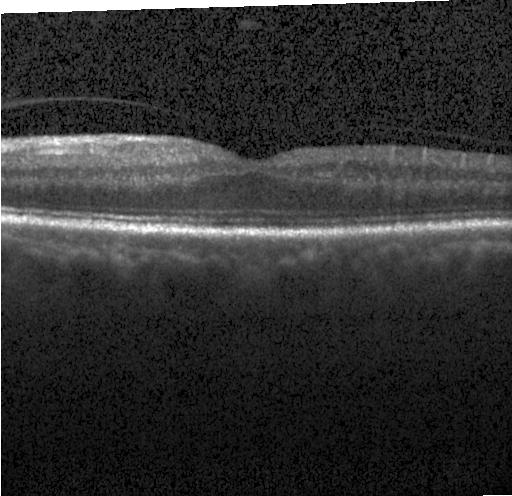 SD-OCT. Retinal OCT B-scan
OCT finding: neither choroidal neovascularization, diabetic macular edema, nor drusen.